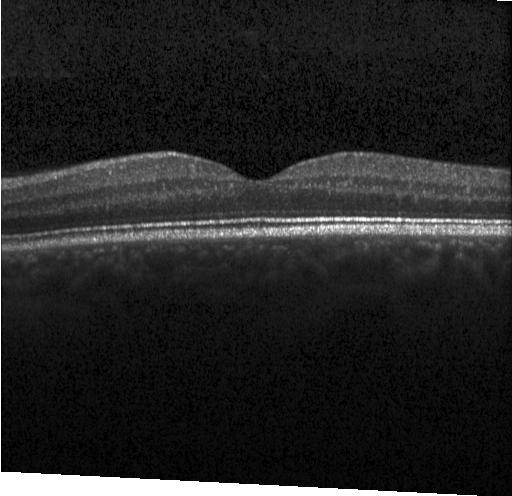

OCT line scan — Diagnosis: no choroidal neovascularization, no diabetic macular edema, and no drusen.